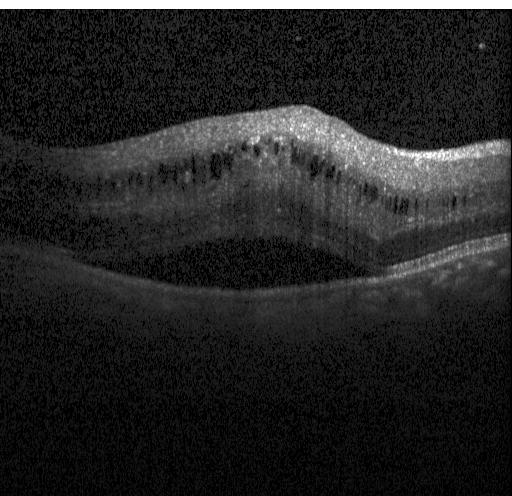

Optical coherence tomography B-scan
Finding: DME.